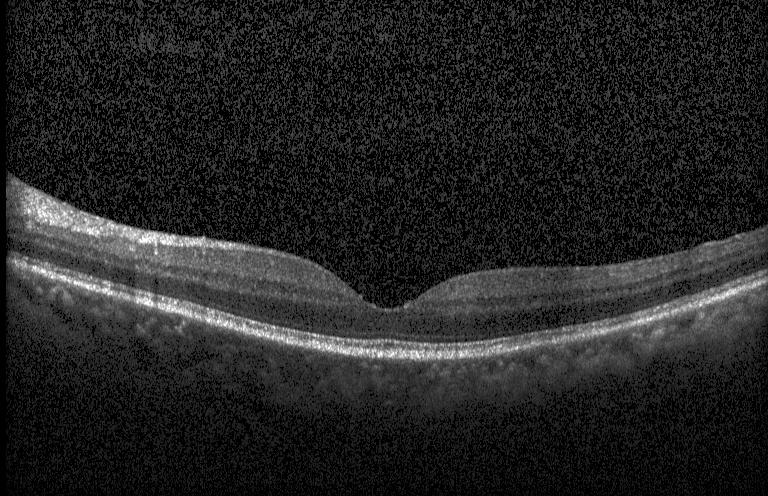 OCT line scan. Diagnosis: no evidence of CNV, DME, or drusen.